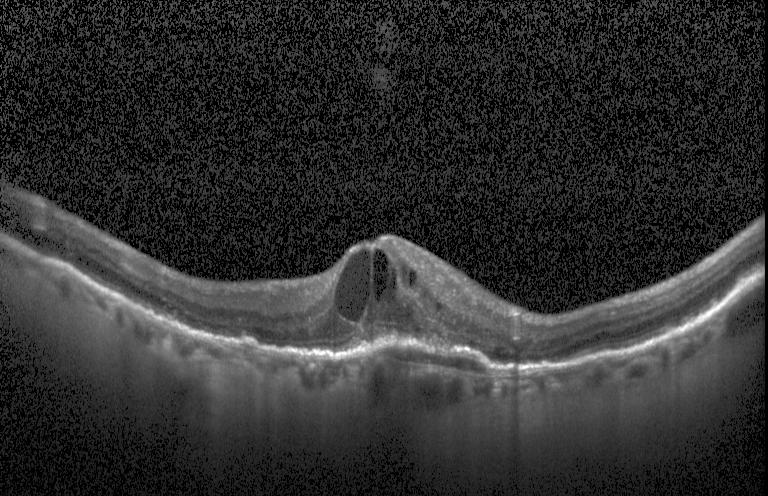
Finding: CNV.